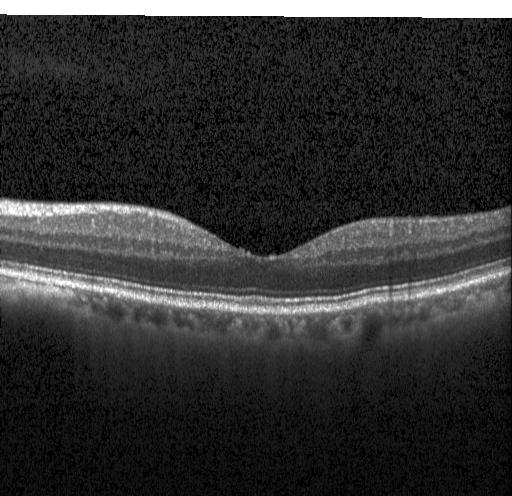 Heidelberg Spectralis · OCT B-scan. Diagnosis: no choroidal neovascularization, diabetic macular edema, or drusen.